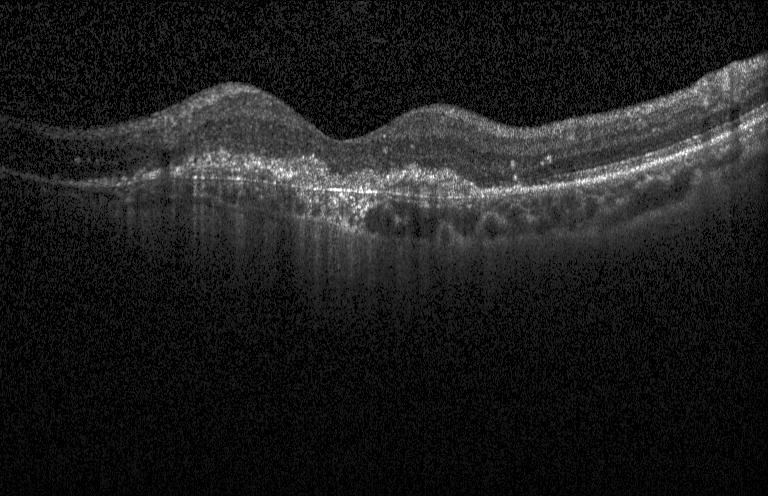

OCT B-scan showing a choroidal neovascular membrane.